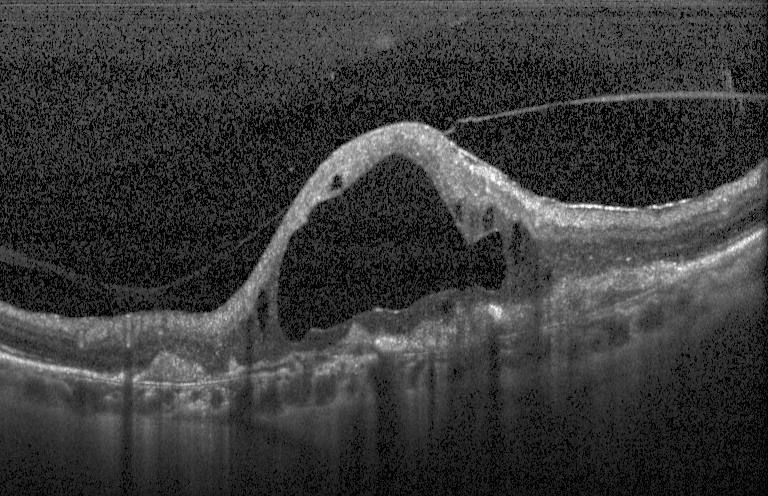

Spectral-domain OCT. OCT B-scan
Assessment: a choroidal neovascular membrane.